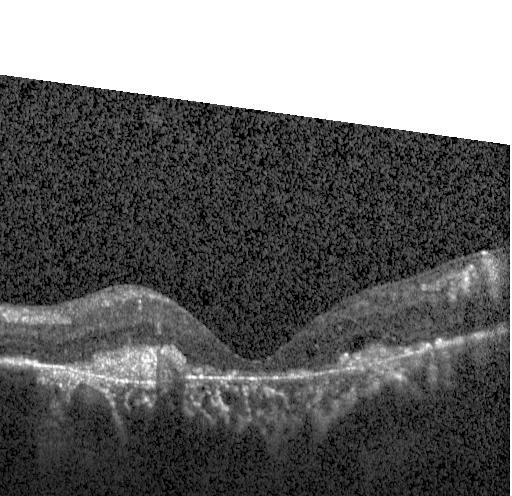

Retinal OCT B-scan
The scan shows choroidal neovascularization (CNV).